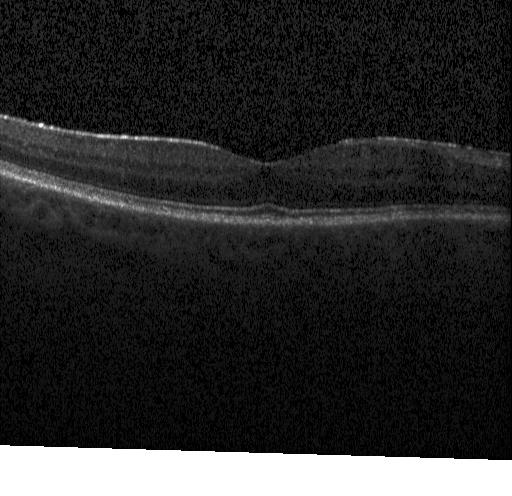 Optical coherence tomography B-scan. Finding: neither choroidal neovascularization, diabetic macular edema, nor drusen.